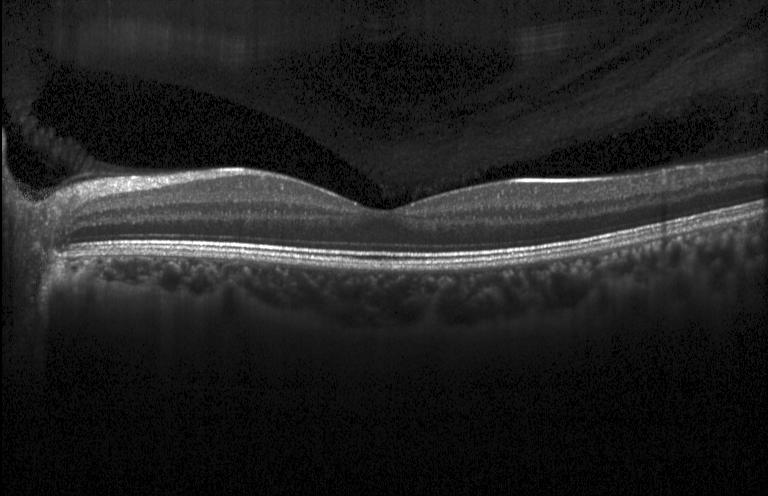 Spectral-domain optical coherence tomography. Optical coherence tomography B-scan
Impression: neither choroidal neovascularization, diabetic macular edema, nor drusen.